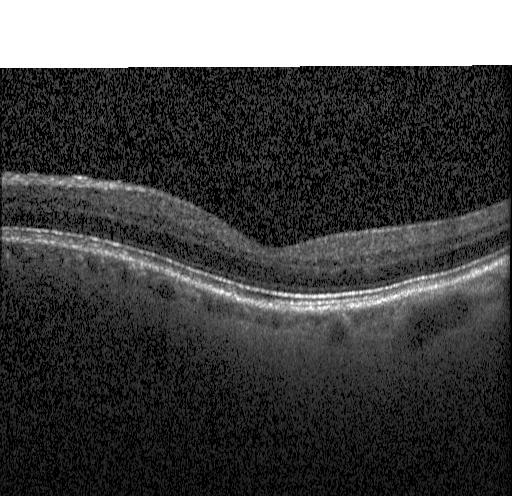

Heidelberg Spectralis OCT system, retinal OCT B-scan, centered on the fovea, spectral-domain optical coherence tomography.
Impression: no choroidal neovascularization, no diabetic macular edema, and no drusen.